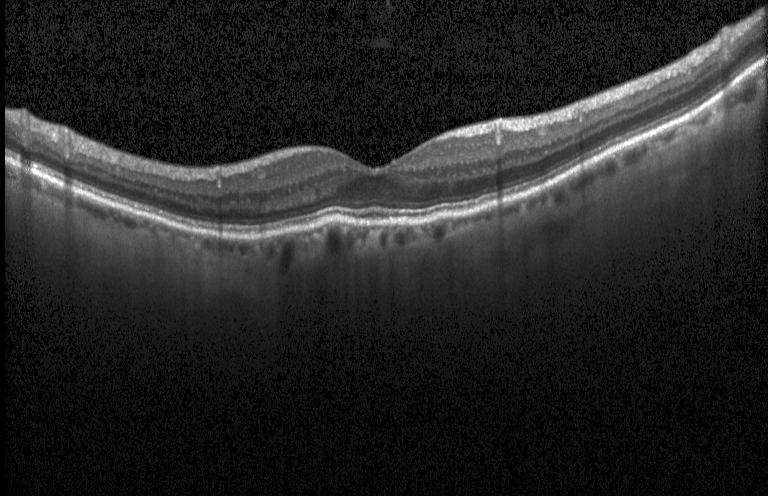
Macular OCT demonstrating no evidence of CNV, DME, or drusen.